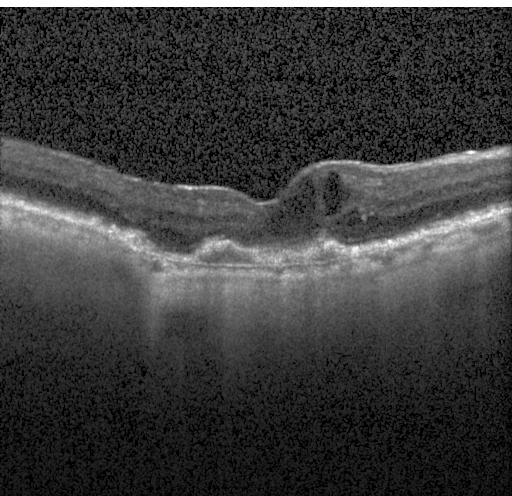

OCT scan showing a choroidal neovascular membrane.